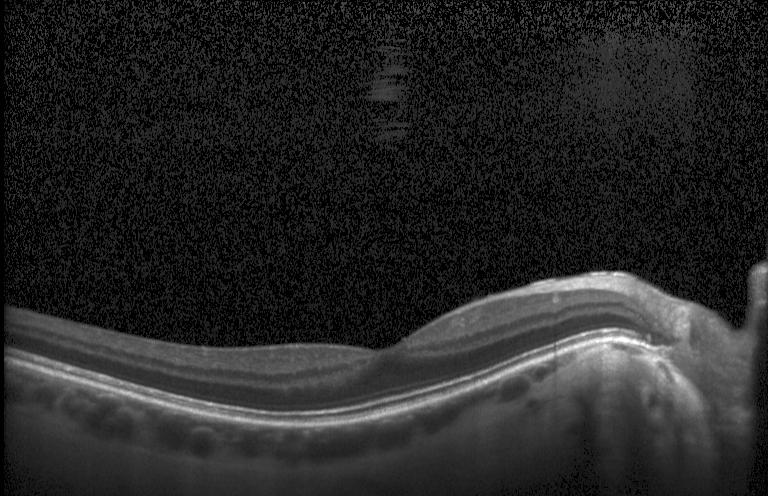

Retinal OCT B-scan, SD-OCT — OCT finding: no choroidal neovascularization, diabetic macular edema, or drusen.